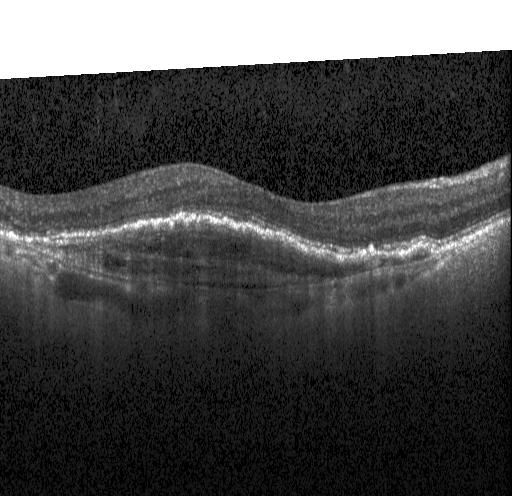
Retinal OCT cross-section showing choroidal neovascularization (CNV).